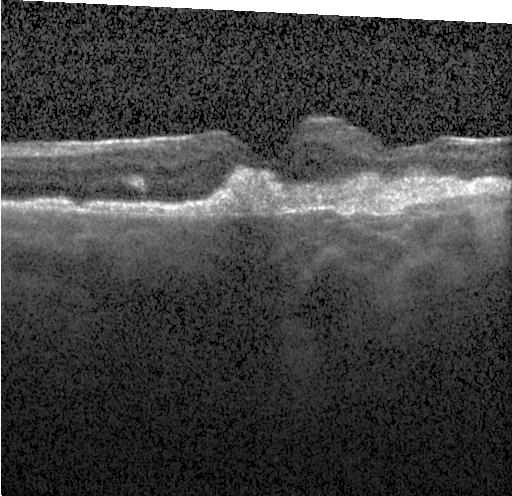
Retinal OCT B-scan.
Diagnosis: a choroidal neovascular membrane.